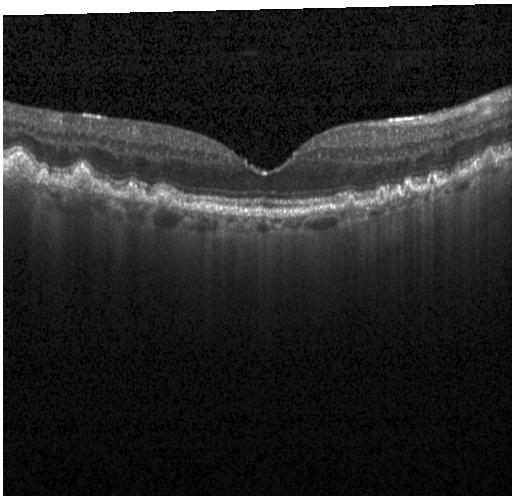 Multiple drusen.